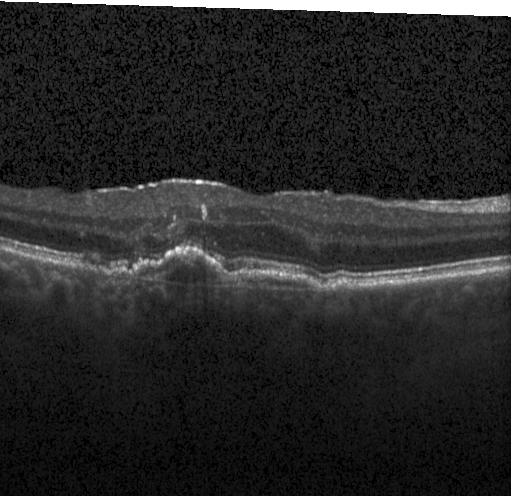
Retinal OCT B-scan; spectral-domain OCT; instrument: Heidelberg Spectralis — Impression: a choroidal neovascular membrane.